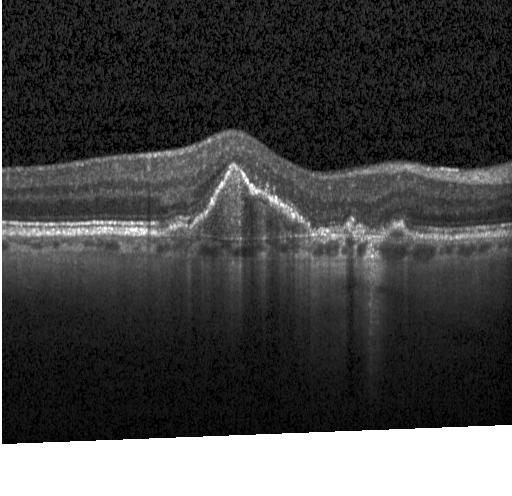
Instrument: Heidelberg Spectralis; OCT B-scan — Dx: a choroidal neovascular membrane.